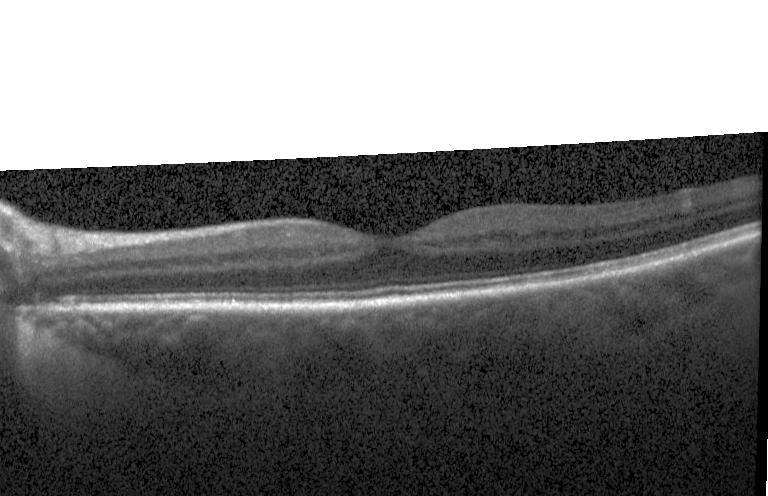
Through the macula. SD-OCT. Instrument: Heidelberg Spectralis. Retinal OCT B-scan.
Assessment: no CNV, no DME, and no drusen.